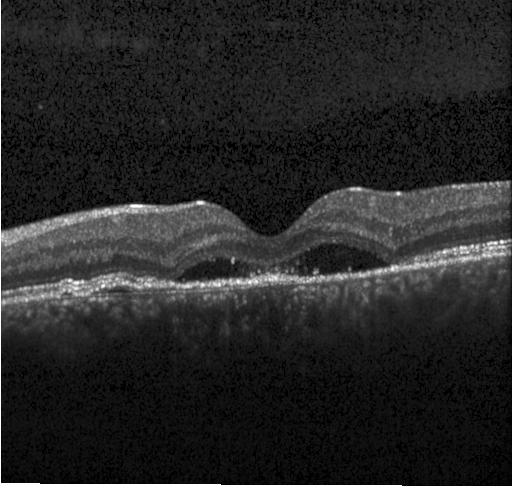 Acquired on a Heidelberg Spectralis, spectral-domain OCT, OCT line scan — Diagnosis: choroidal neovascularization.